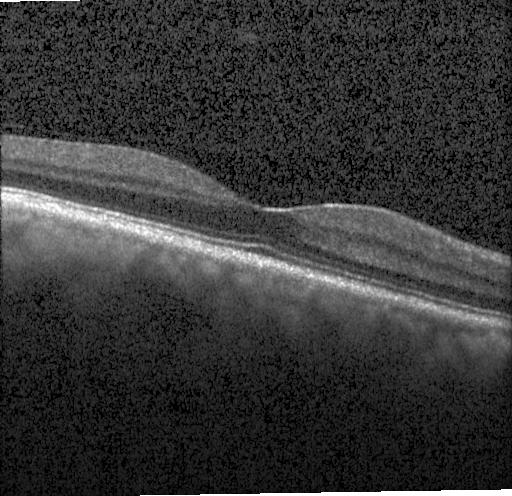
OCT B-scan.
Dx: no evidence of choroidal neovascularization, diabetic macular edema, or drusen.